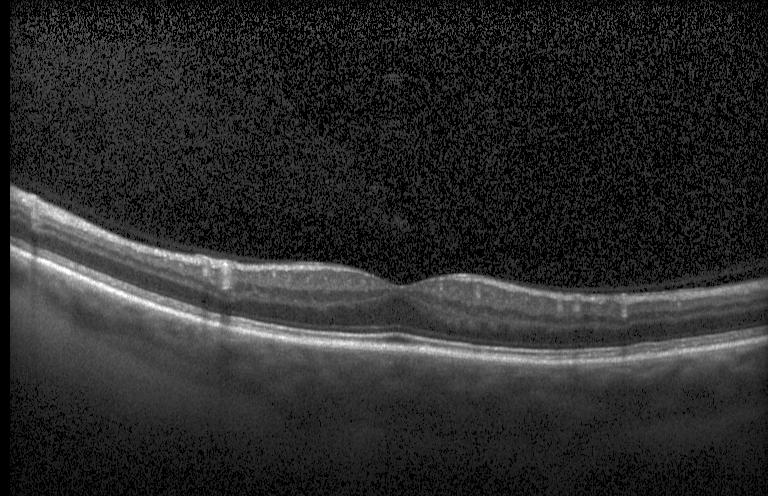

Retinal OCT cross-section showing no evidence of choroidal neovascularization, diabetic macular edema, or drusen.